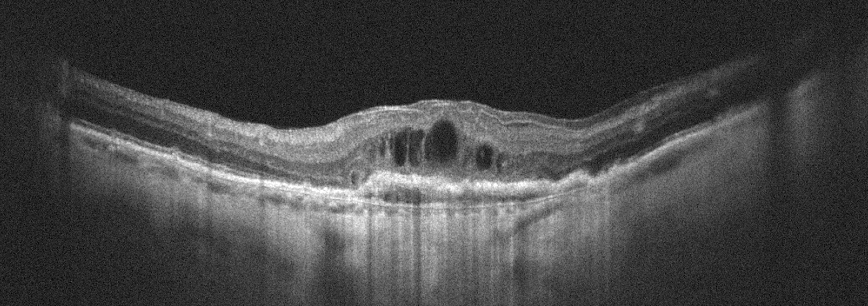

OCT line scan; instrument: Optovue Avanti RTVue XR — Finding: age-related macular degeneration.